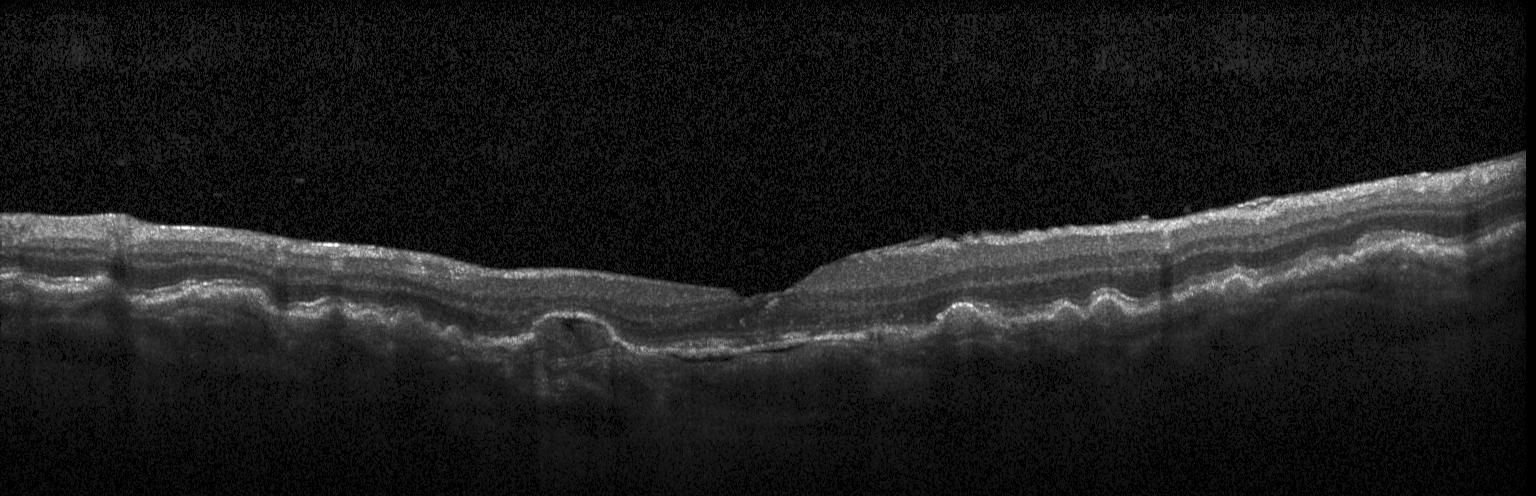 Heidelberg Spectralis · optical coherence tomography scan — This B-scan demonstrates a choroidal neovascular membrane.